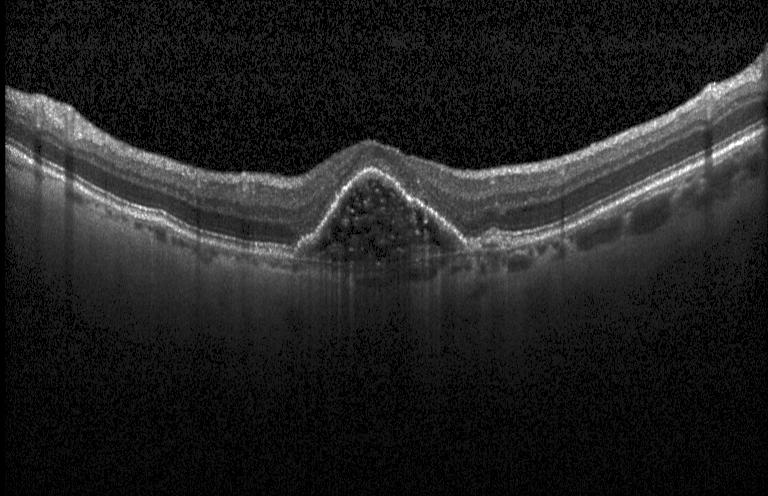 Dx: choroidal neovascularization (CNV).